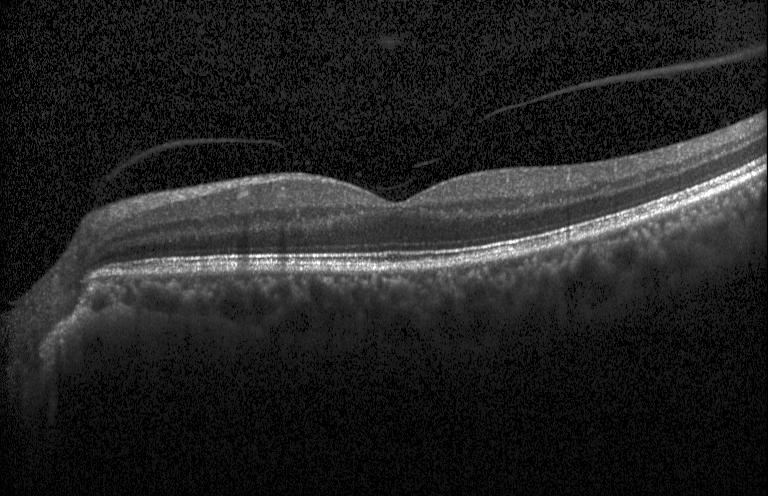
Optical coherence tomography B-scan, Heidelberg Spectralis. OCT finding: no evidence of choroidal neovascularization, diabetic macular edema, or drusen.